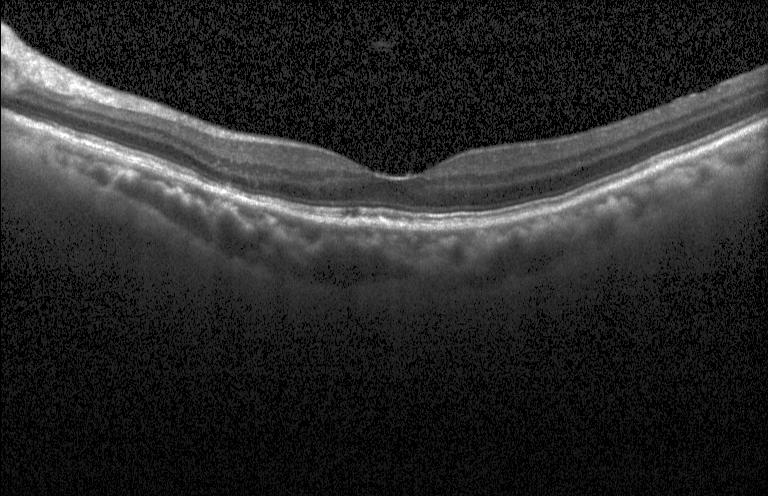

Impression: neither choroidal neovascularization, diabetic macular edema, nor drusen.